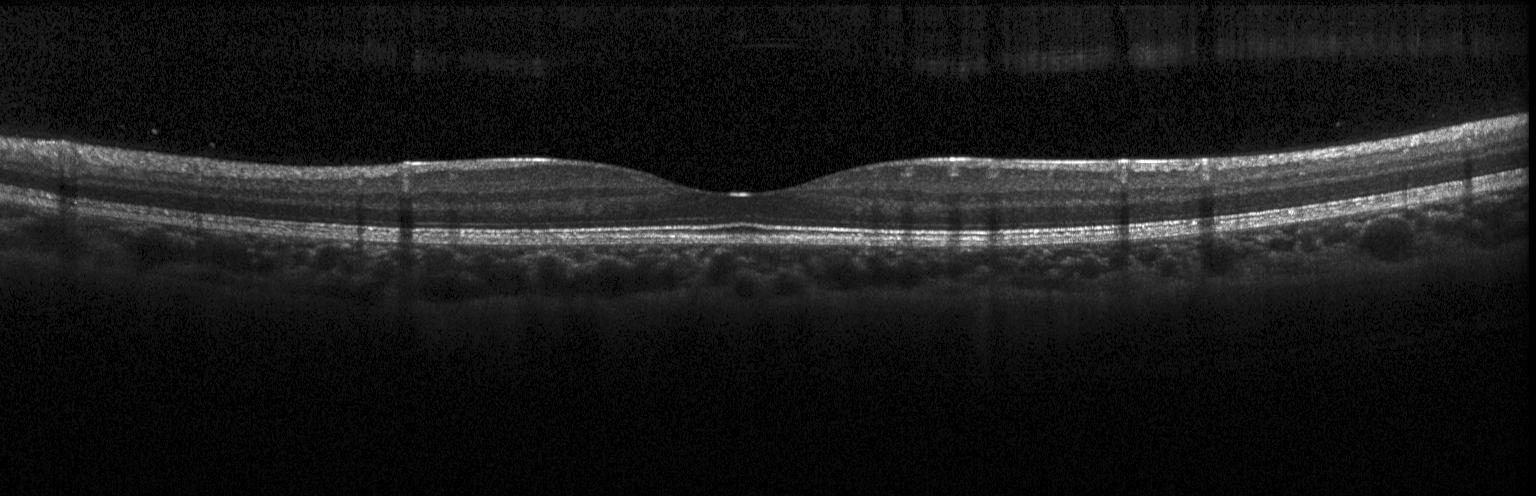
OCT B-scan · Heidelberg Spectralis
This B-scan demonstrates no evidence of CNV, DME, or drusen.